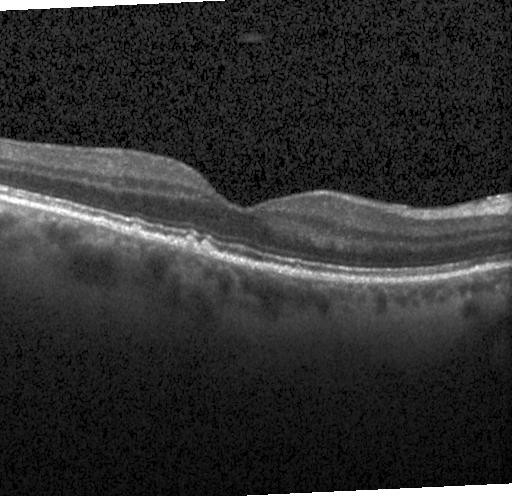
Spectral-domain OCT · horizontal scan through the fovea · retinal OCT B-scan
This B-scan demonstrates sub-RPE drusenoid deposits.